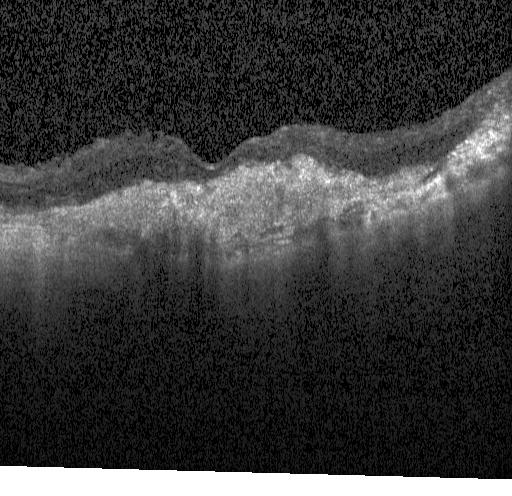 This B-scan demonstrates choroidal neovascularization (CNV).